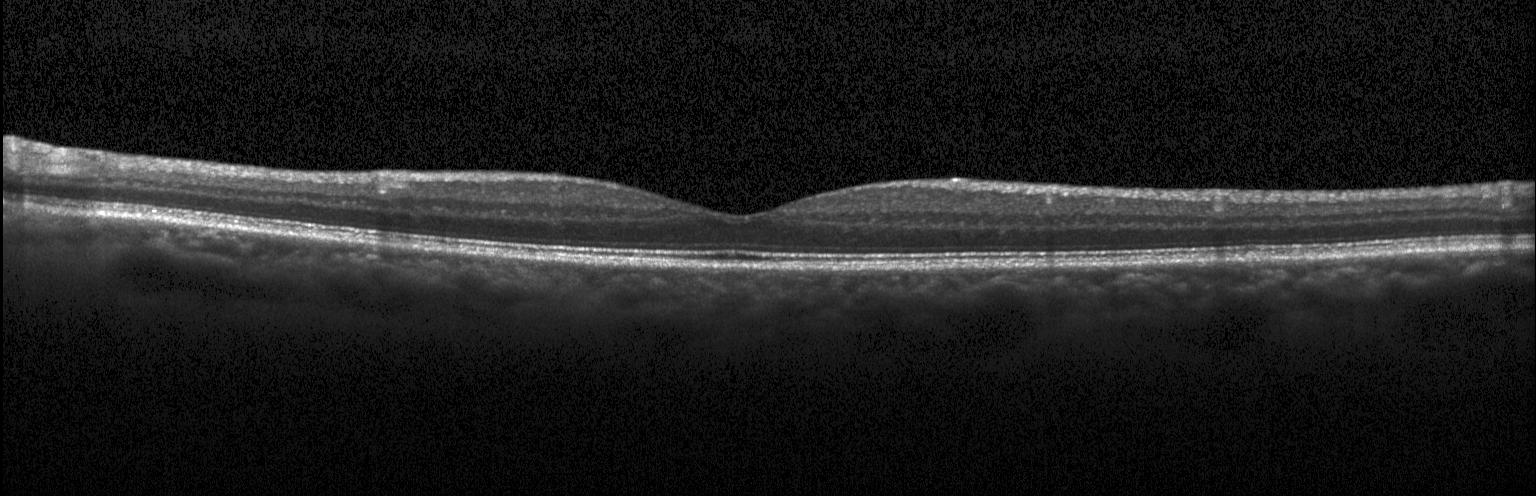 Impression: no choroidal neovascularization, no diabetic macular edema, and no drusen.